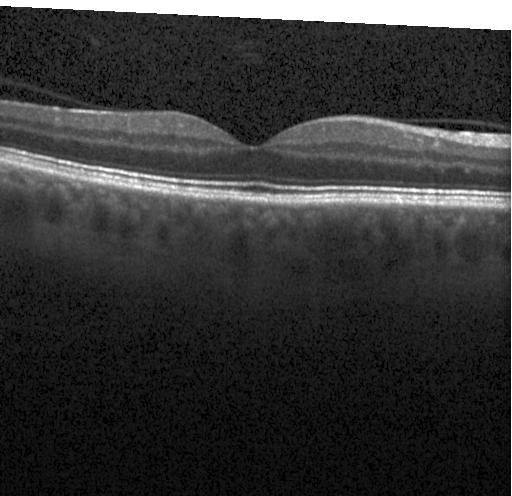
Retinal OCT B-scan · horizontal scan through the fovea · SD-OCT — This B-scan demonstrates no evidence of CNV, DME, or drusen.